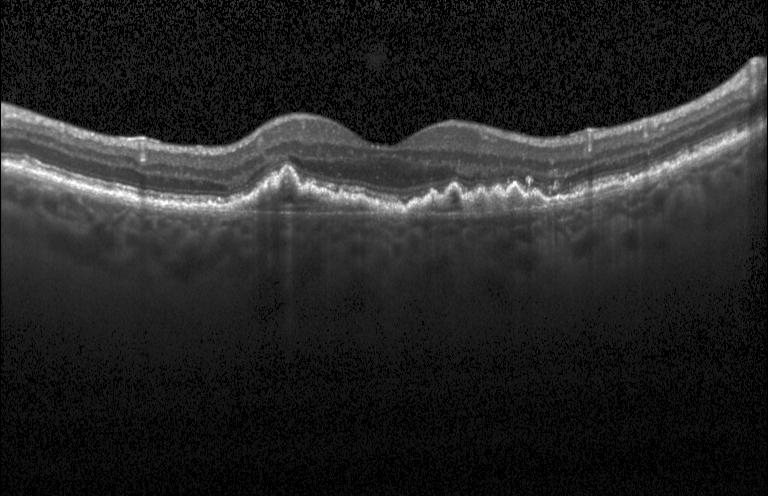 SD-OCT. Macular scan. Retinal OCT cross-section. Acquired on a Heidelberg Spectralis
CNV.